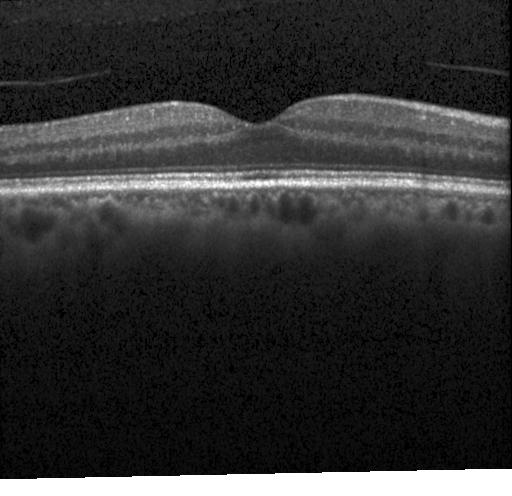
Optical coherence tomography scan, centered on the fovea, acquired on a Heidelberg Spectralis
Finding: neither CNV, DME, nor drusen.